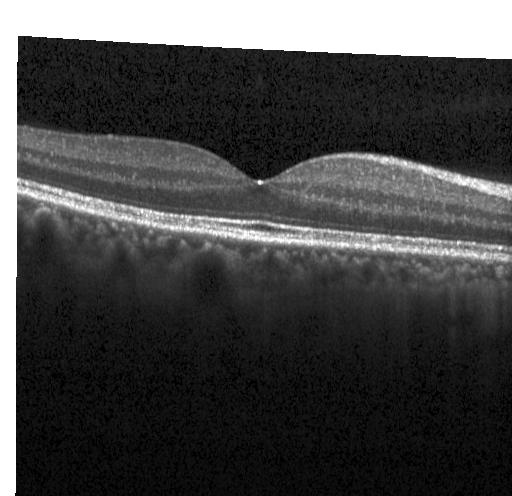
Spectral-domain OCT · OCT B-scan — Finding: neither CNV, DME, nor drusen.